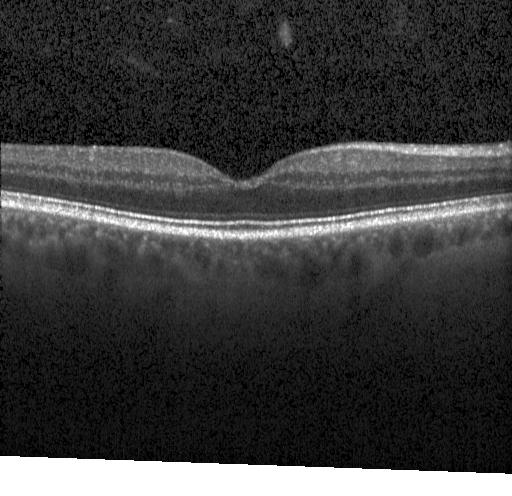

This B-scan demonstrates no evidence of choroidal neovascularization, diabetic macular edema, or drusen.